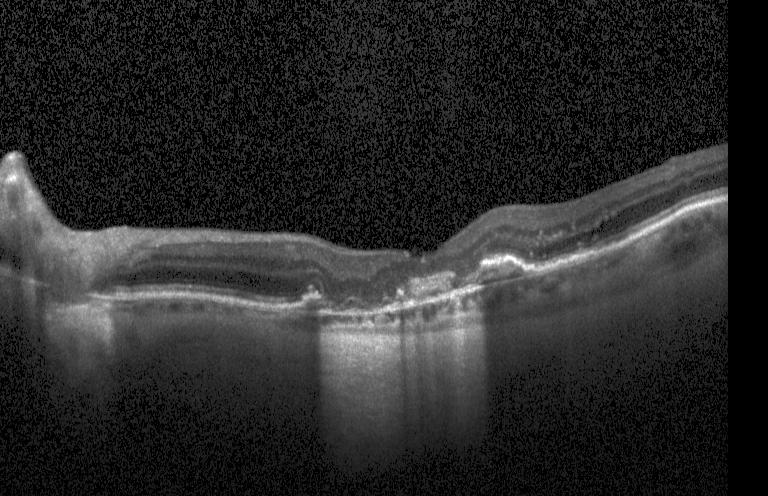 CNV.